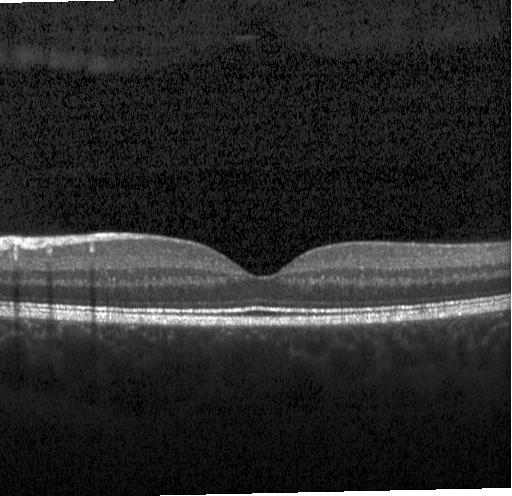
Spectral-domain optical coherence tomography; OCT B-scan; through the macula. Assessment: neither choroidal neovascularization, diabetic macular edema, nor drusen.